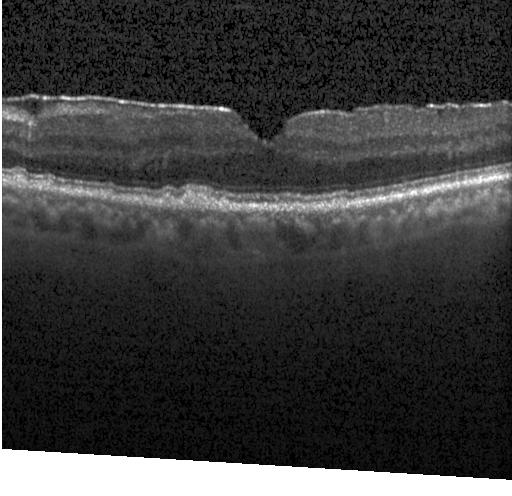 OCT line scan; Heidelberg Spectralis.
Finding: sub-RPE drusenoid deposits.